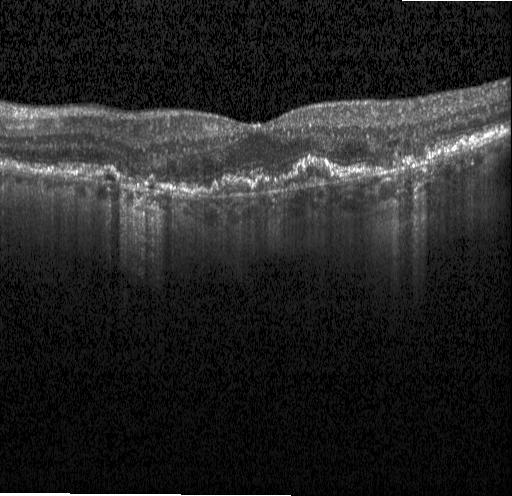
Horizontal scan through the fovea · optical coherence tomography scan
Dx: a choroidal neovascular membrane.